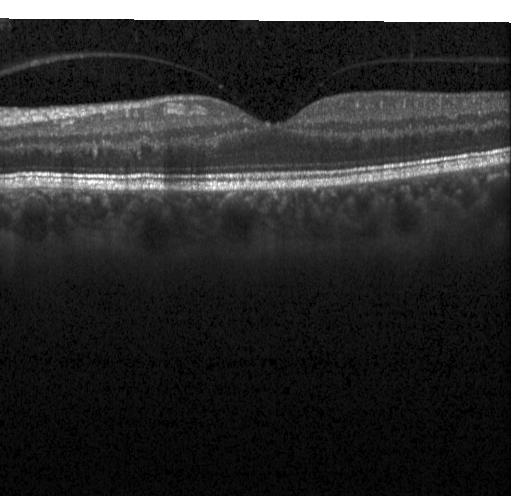 Impression: no choroidal neovascularization, diabetic macular edema, or drusen.